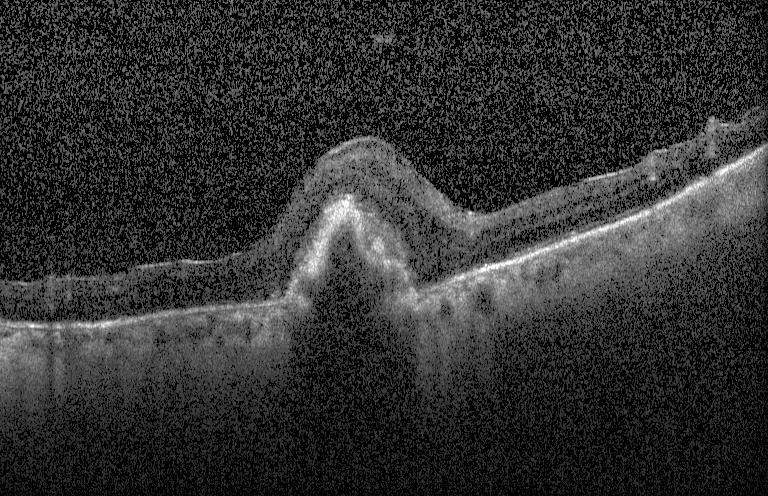

This B-scan demonstrates choroidal neovascularization (CNV).